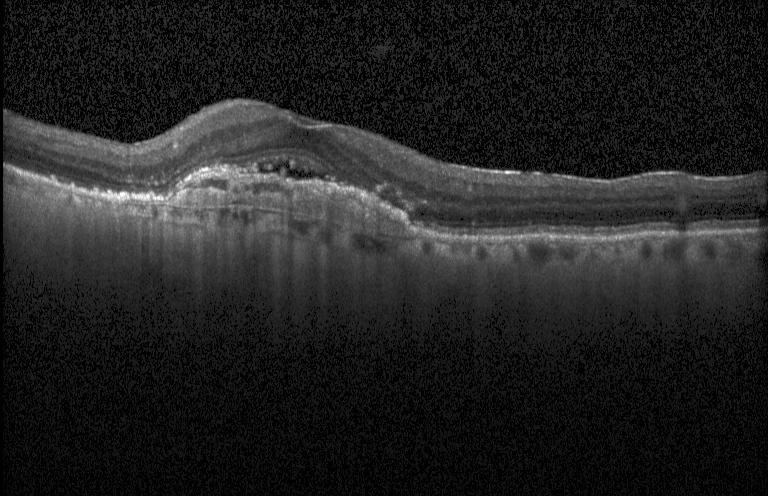 Through the macula · SD-OCT · Heidelberg Spectralis · optical coherence tomography B-scan.
Impression: choroidal neovascularization.